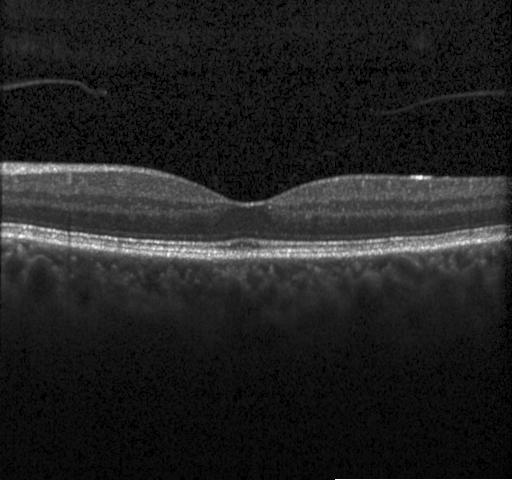
OCT B-scan showing no evidence of choroidal neovascularization, diabetic macular edema, or drusen.